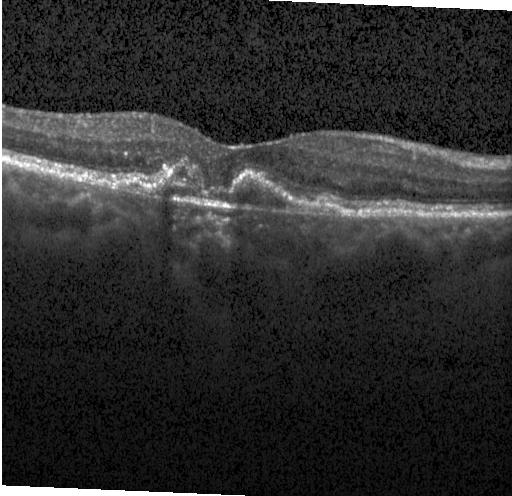
OCT B-scan. Finding: a choroidal neovascular membrane.